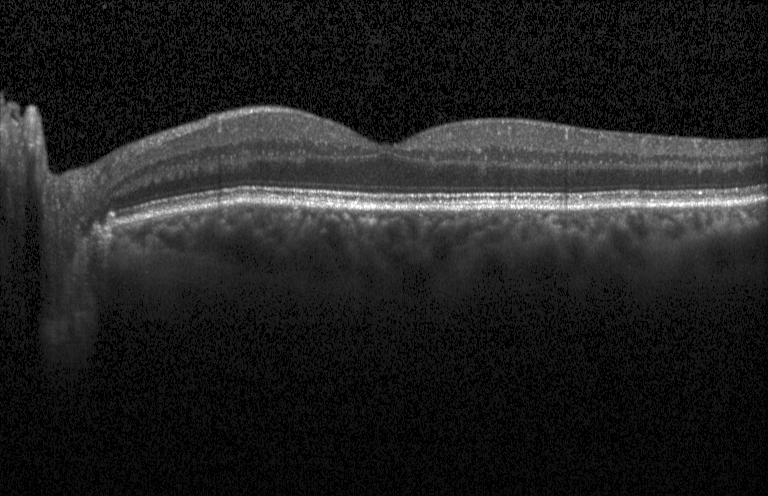 Finding: no evidence of choroidal neovascularization, diabetic macular edema, or drusen.